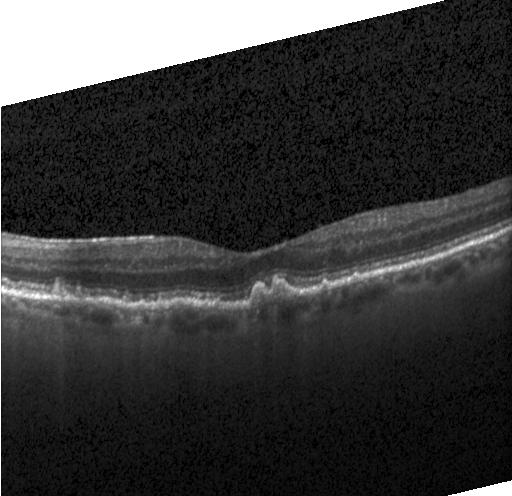
Retinal OCT cross-section showing sub-RPE drusenoid deposits.